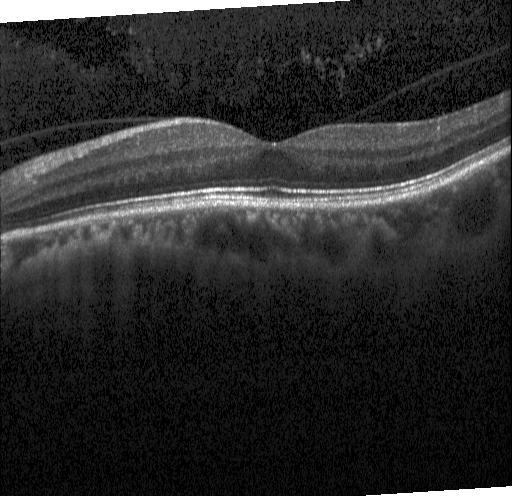
Optical coherence tomography B-scan. The scan shows no evidence of CNV, DME, or drusen.